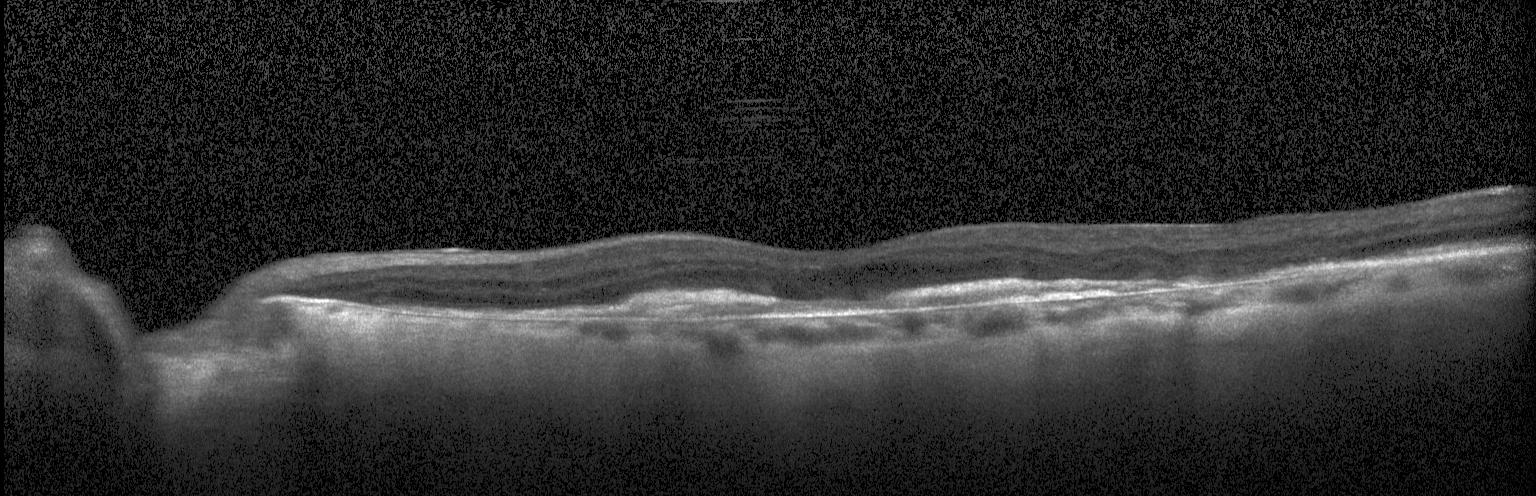 Finding: a choroidal neovascular membrane.